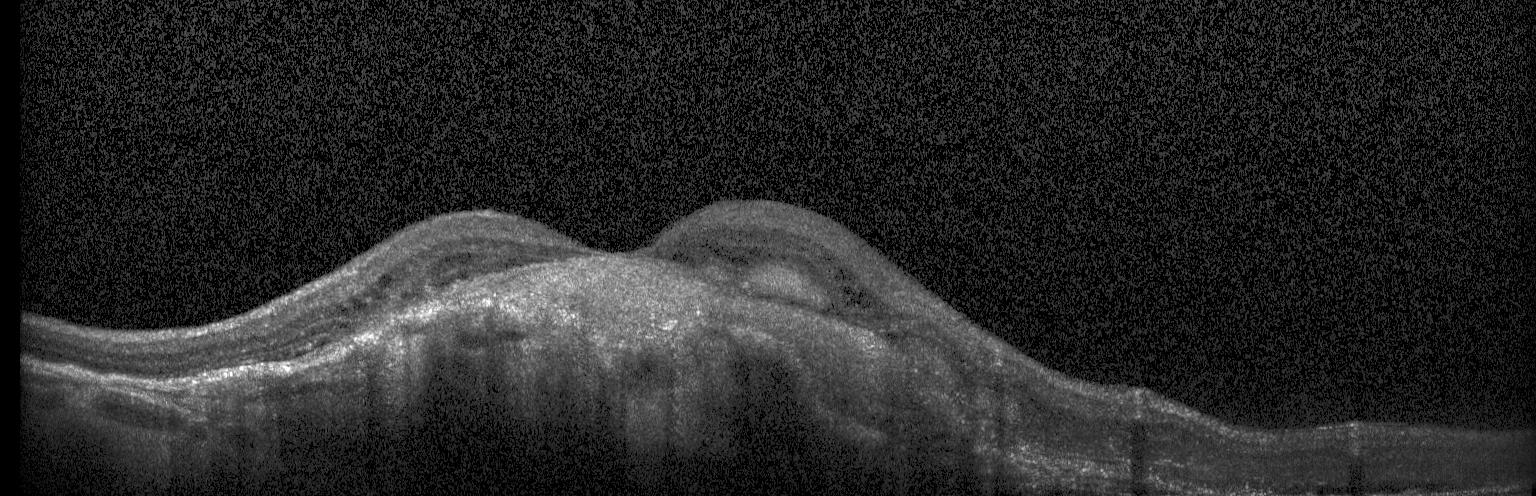 Optical coherence tomography B-scan — Macular OCT: choroidal neovascularization.